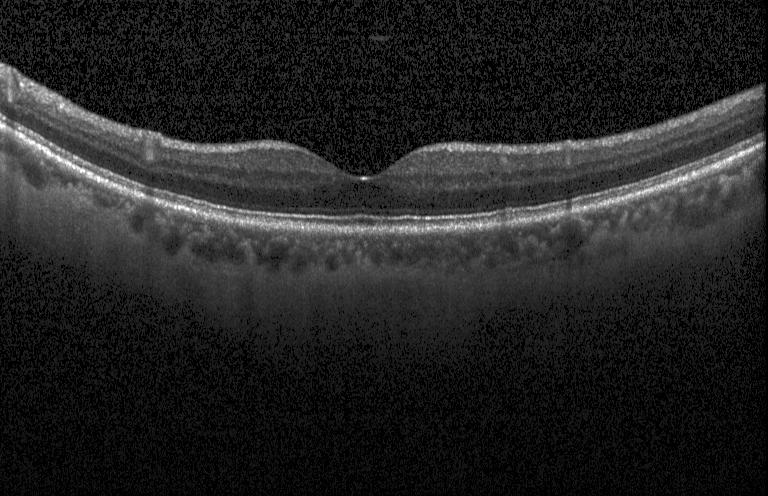
Heidelberg Spectralis, spectral-domain OCT, optical coherence tomography B-scan, macular scan — Diagnosis: neither CNV, DME, nor drusen.